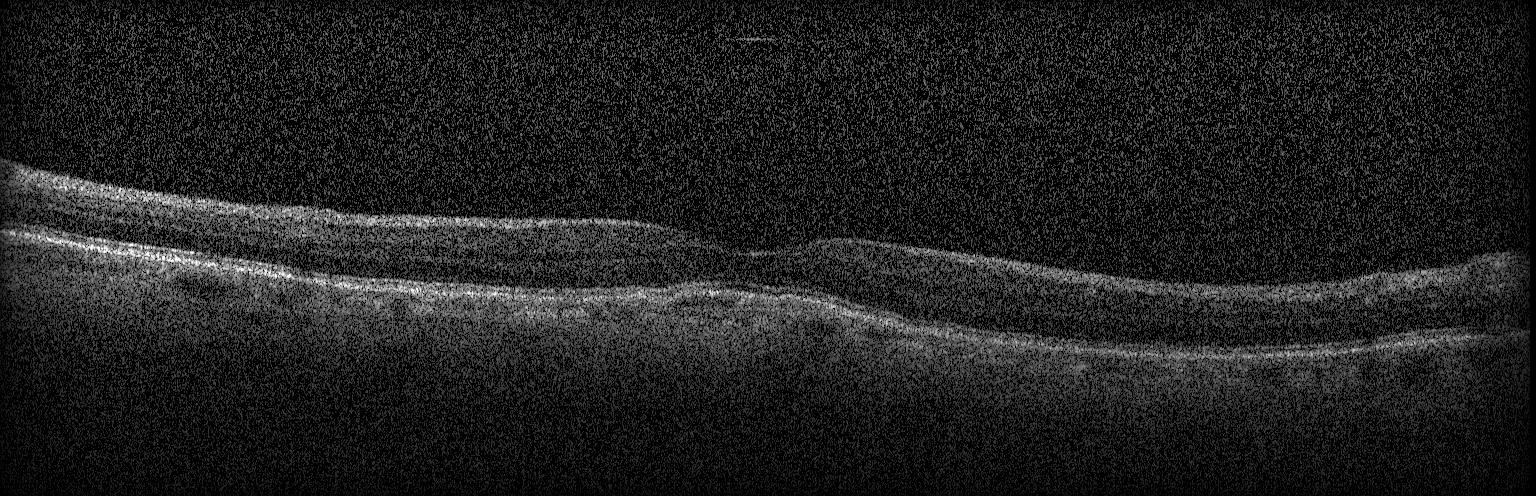
Impression: a choroidal neovascular membrane.